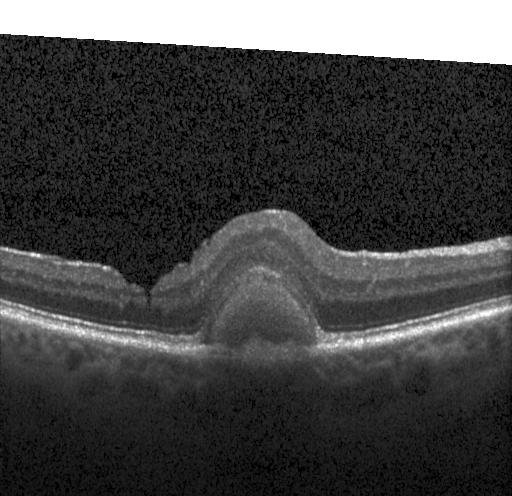 Heidelberg Spectralis, SD-OCT, retinal OCT cross-section, fovea-centered — The scan shows CNV.